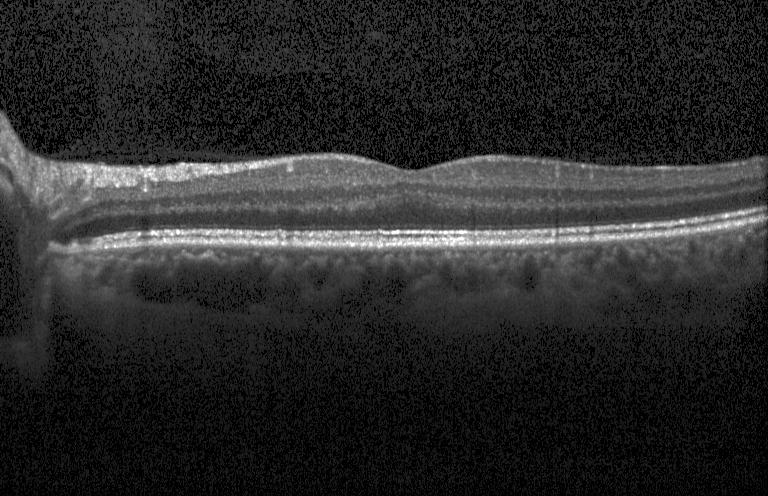
Heidelberg Spectralis OCT system; retinal OCT B-scan
Macular OCT: no evidence of choroidal neovascularization, diabetic macular edema, or drusen.